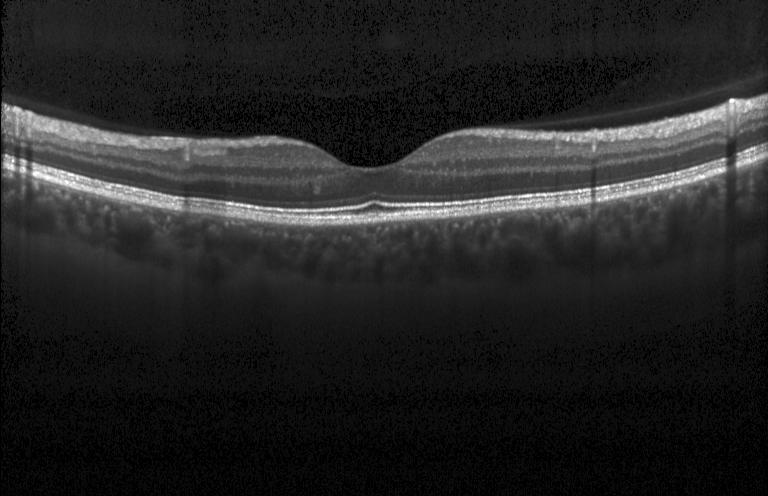 Retinal OCT cross-section; SD-OCT; Heidelberg Spectralis; fovea-centered — OCT finding: no choroidal neovascularization, no diabetic macular edema, and no drusen.